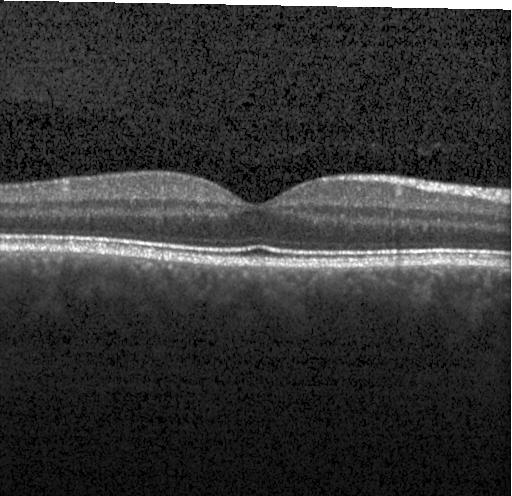

Heidelberg Spectralis OCT system, optical coherence tomography scan, fovea-centered, spectral-domain optical coherence tomography.
Finding: no evidence of choroidal neovascularization, diabetic macular edema, or drusen.